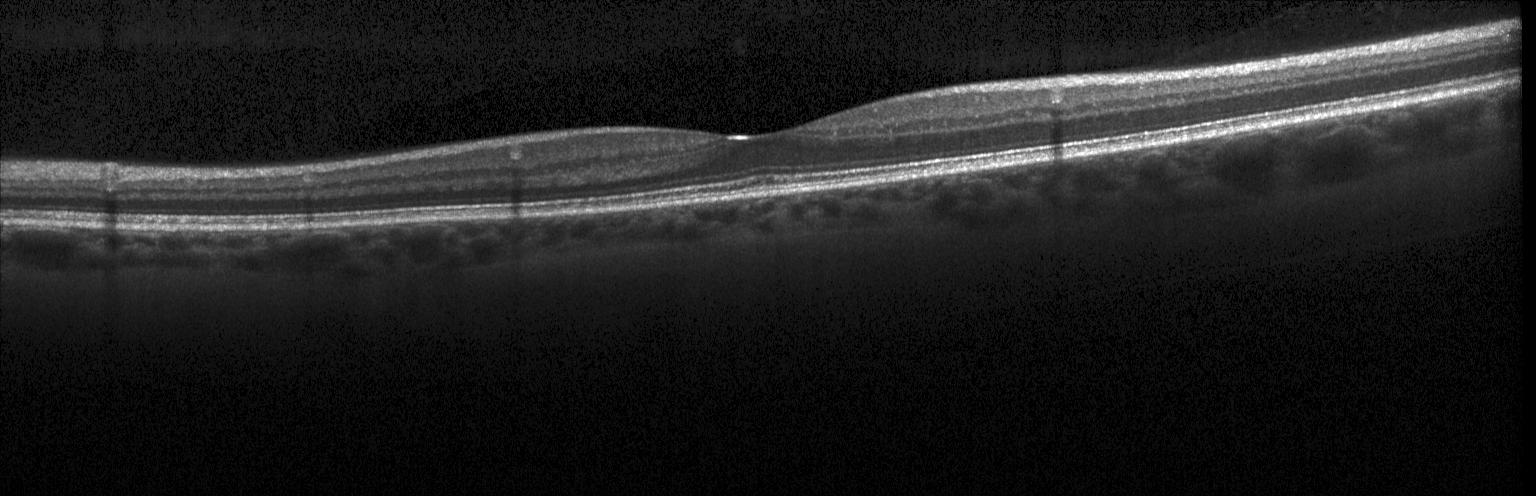 Retinal OCT cross-section showing no choroidal neovascularization, diabetic macular edema, or drusen.